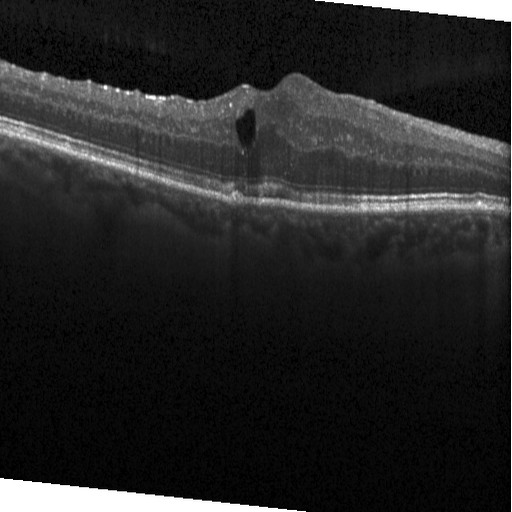 OCT B-scan. OCT finding: diabetic macular edema.